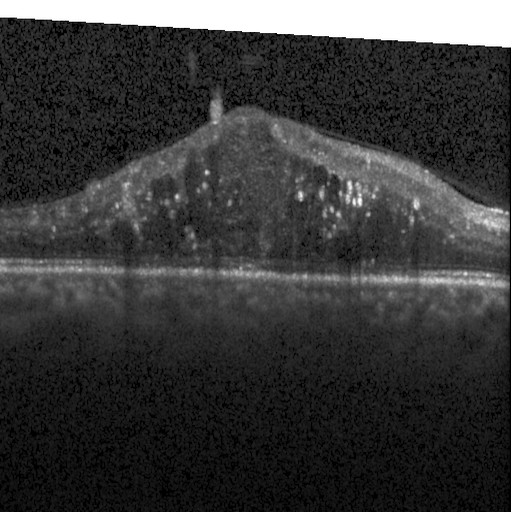 Through the macula. Retinal OCT B-scan. Spectral-domain OCT. Acquired on a Heidelberg Spectralis — Impression: DME.